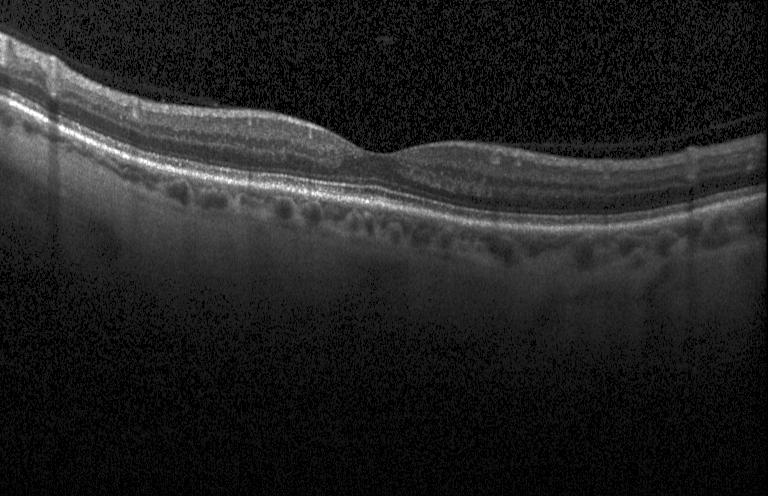
Fovea-centered · Heidelberg Spectralis OCT system · OCT B-scan
Finding: no CNV, DME, or drusen.